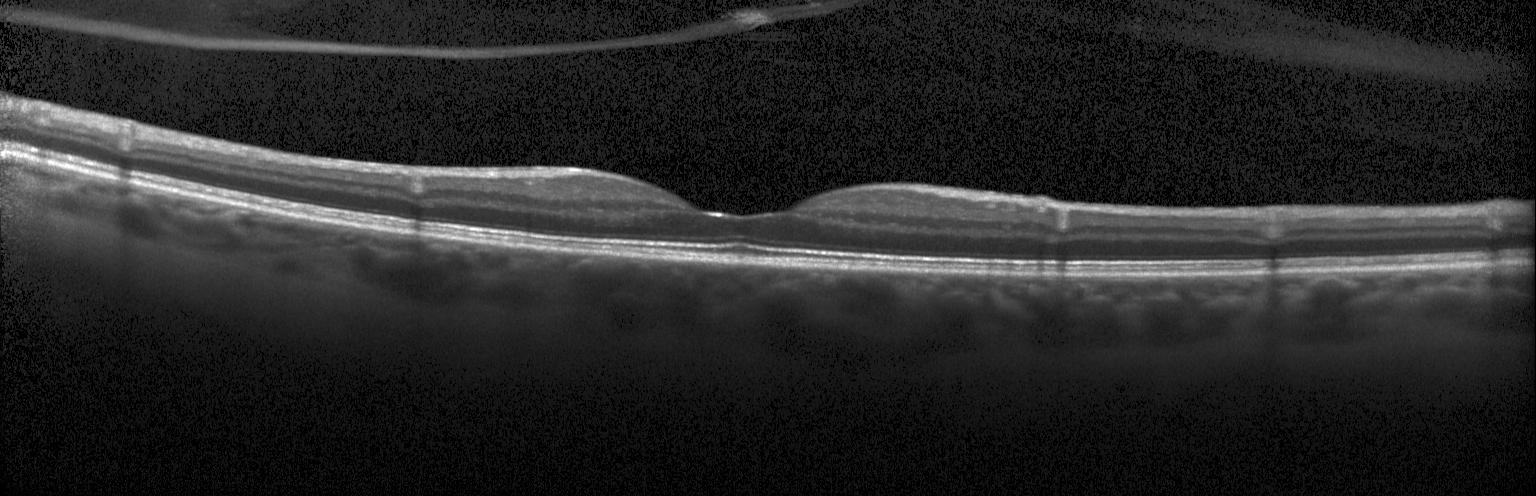

Finding: no choroidal neovascularization, no diabetic macular edema, and no drusen.